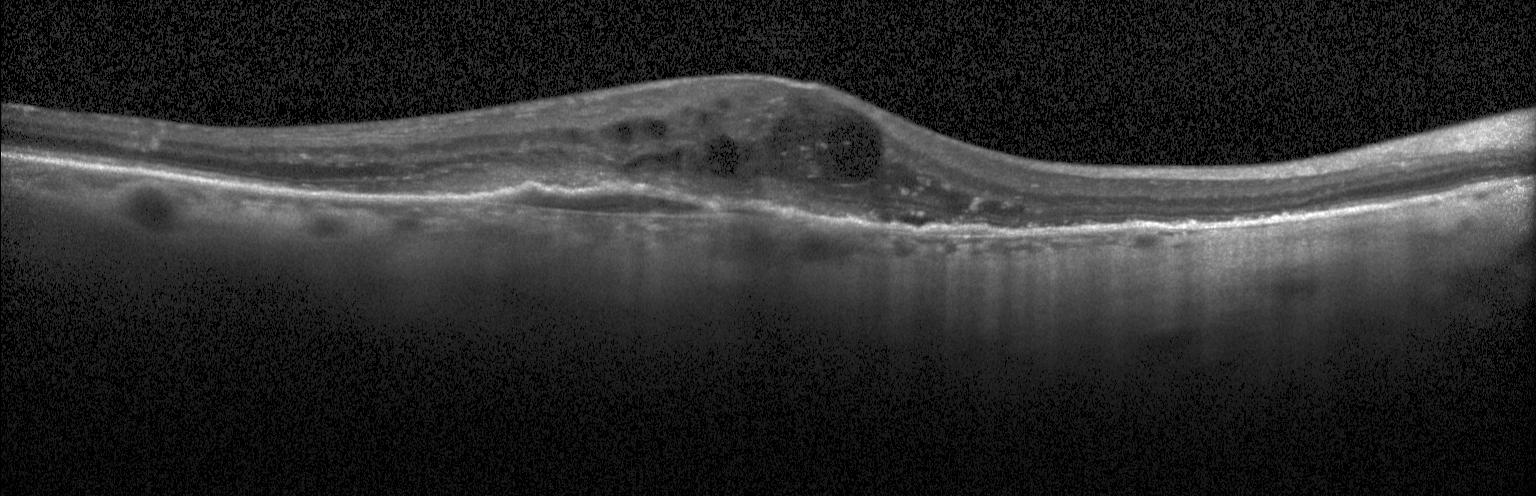 Retinal OCT cross-section; instrument: Heidelberg Spectralis; SD-OCT
Choroidal neovascularization (CNV).